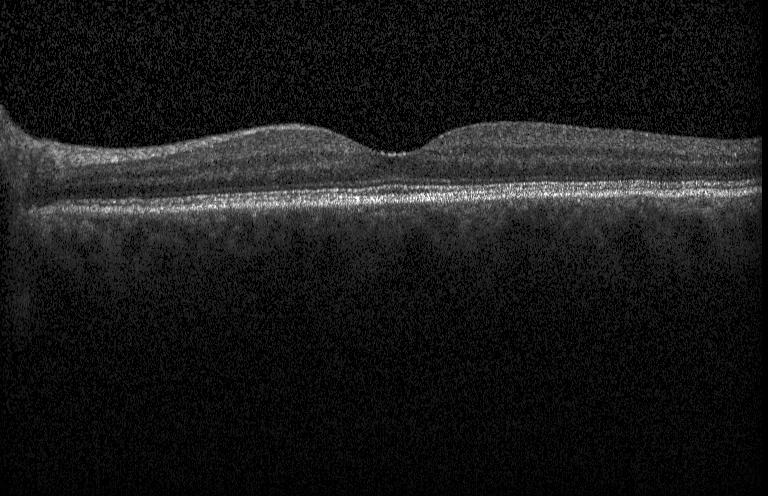
Horizontal scan through the fovea · optical coherence tomography B-scan. Finding: neither choroidal neovascularization, diabetic macular edema, nor drusen.